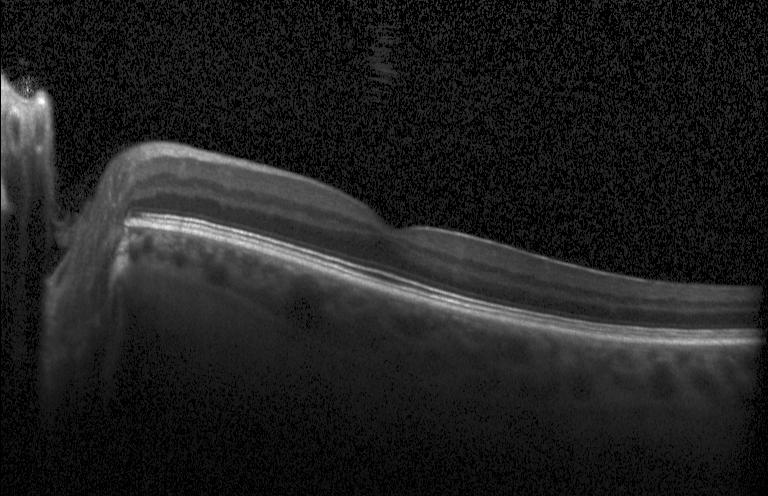
Heidelberg Spectralis OCT system · through the macula · retinal OCT B-scan · SD-OCT. Finding: no evidence of CNV, DME, or drusen.